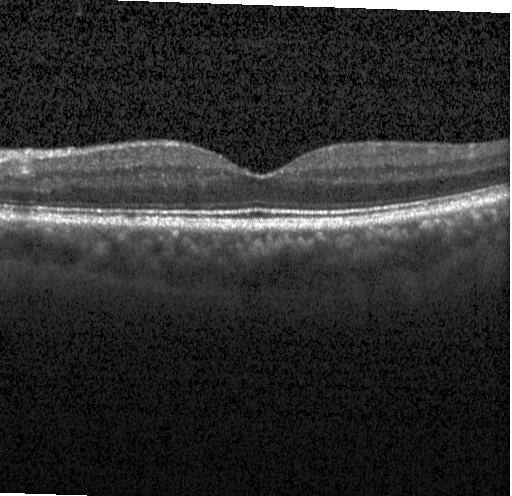 Impression: no evidence of choroidal neovascularization, diabetic macular edema, or drusen.